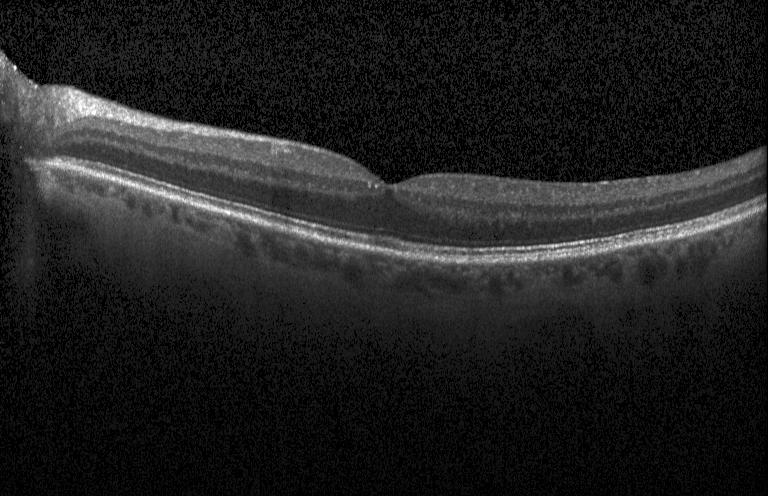

OCT line scan — Diagnosis: no evidence of CNV, DME, or drusen.